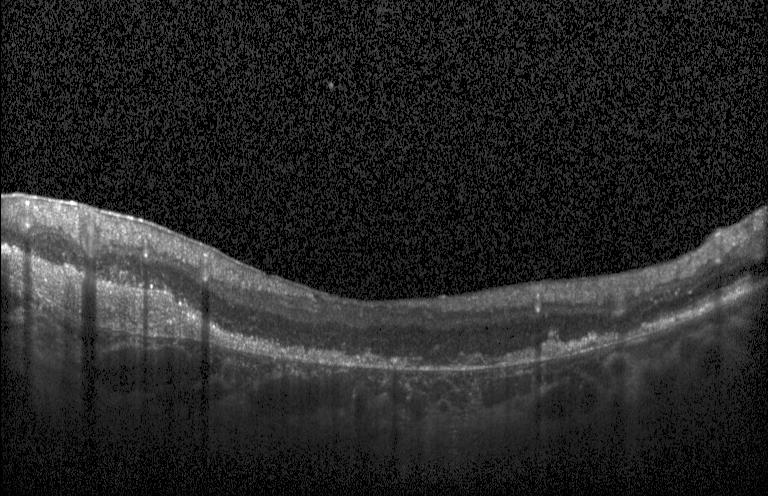

The scan shows a choroidal neovascular membrane.